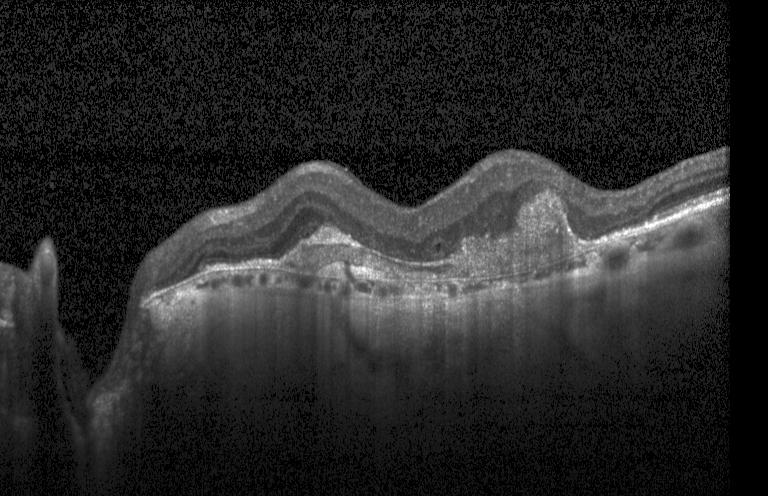

Optical coherence tomography B-scan — Diagnosis: a choroidal neovascular membrane.